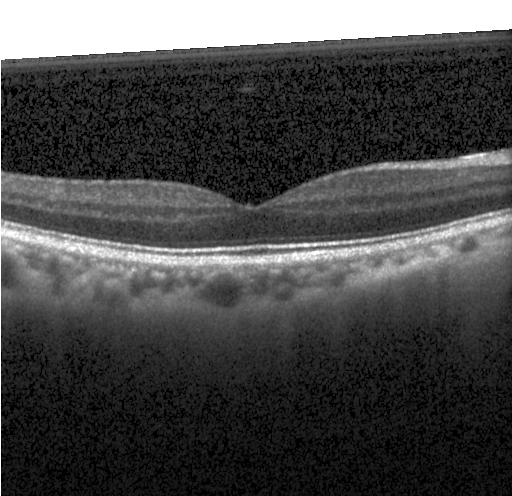 Finding: no choroidal neovascularization, no diabetic macular edema, and no drusen.